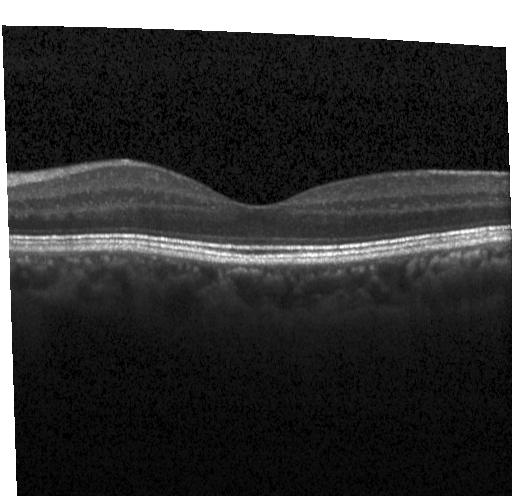 Dx: no evidence of choroidal neovascularization, diabetic macular edema, or drusen.